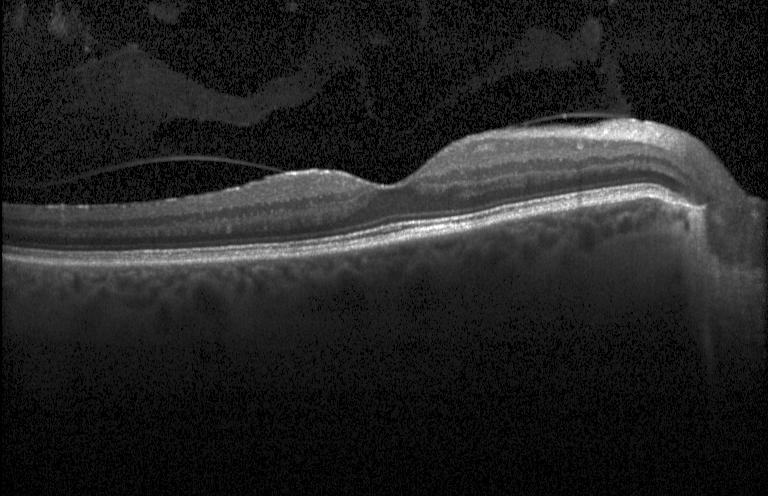

Spectral-domain OCT; optical coherence tomography scan
Finding: no evidence of choroidal neovascularization, diabetic macular edema, or drusen.